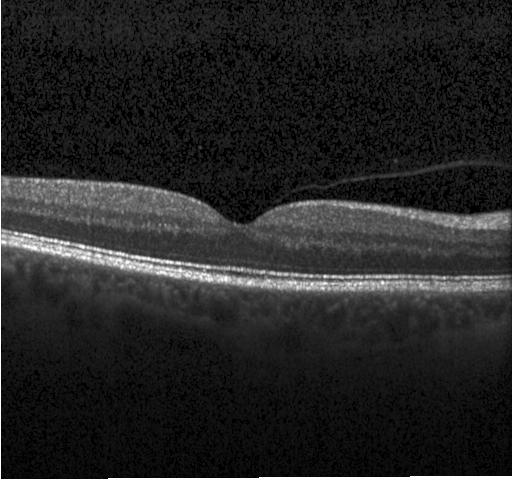 Macular scan, Heidelberg Spectralis, spectral-domain optical coherence tomography, OCT B-scan
Diagnosis: no CNV, DME, or drusen.